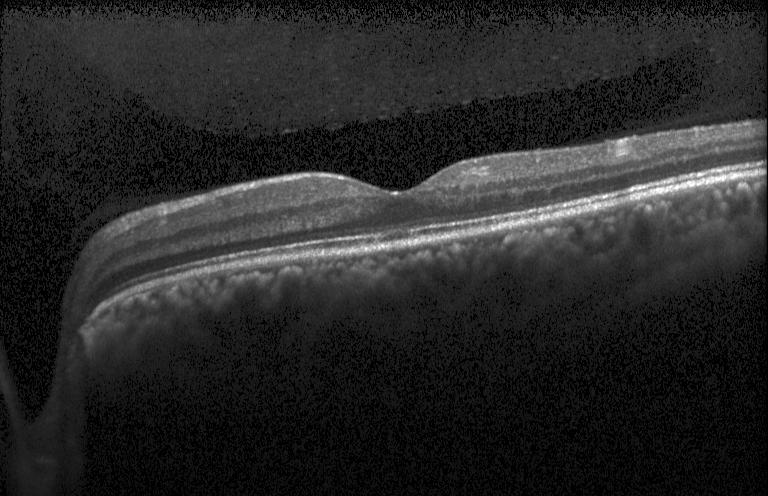
Impression: neither choroidal neovascularization, diabetic macular edema, nor drusen.